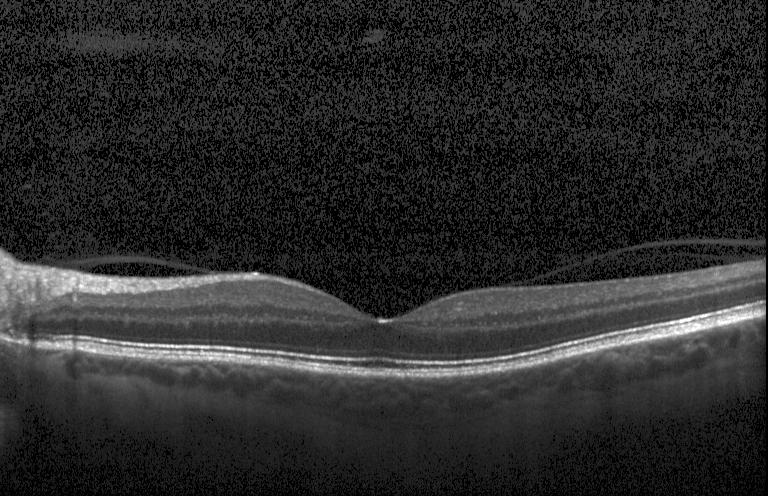
Diagnosis: no CNV, no DME, and no drusen.